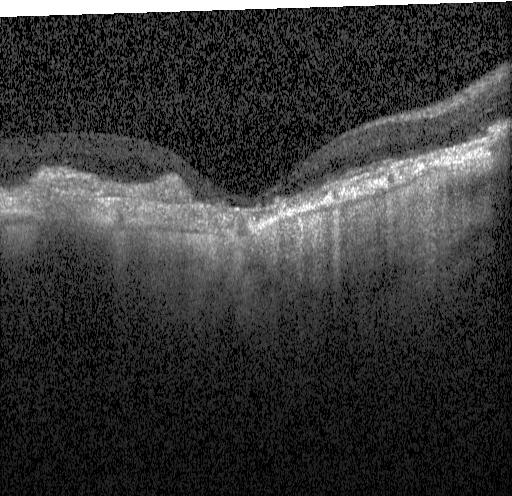 Diagnosis: a choroidal neovascular membrane.